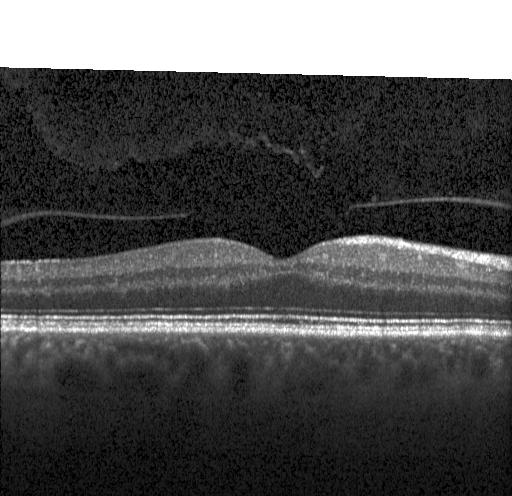

OCT scan showing neither choroidal neovascularization, diabetic macular edema, nor drusen.